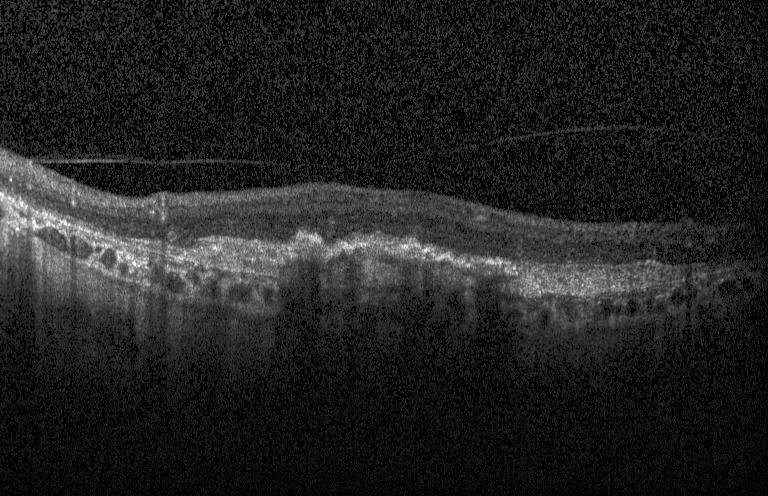

Spectral-domain optical coherence tomography; macular scan; OCT B-scan; instrument: Heidelberg Spectralis. Macular OCT: choroidal neovascularization (CNV).